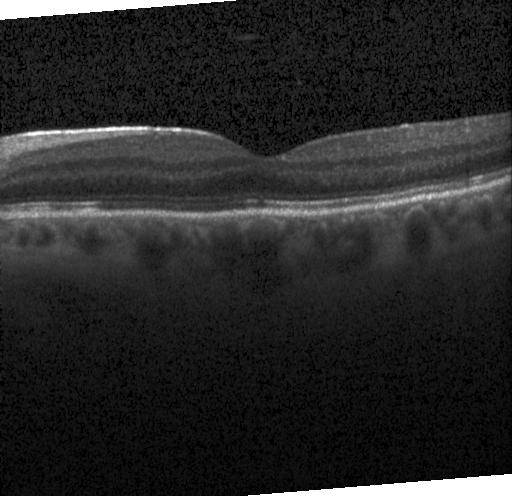 Dx: neither choroidal neovascularization, diabetic macular edema, nor drusen.